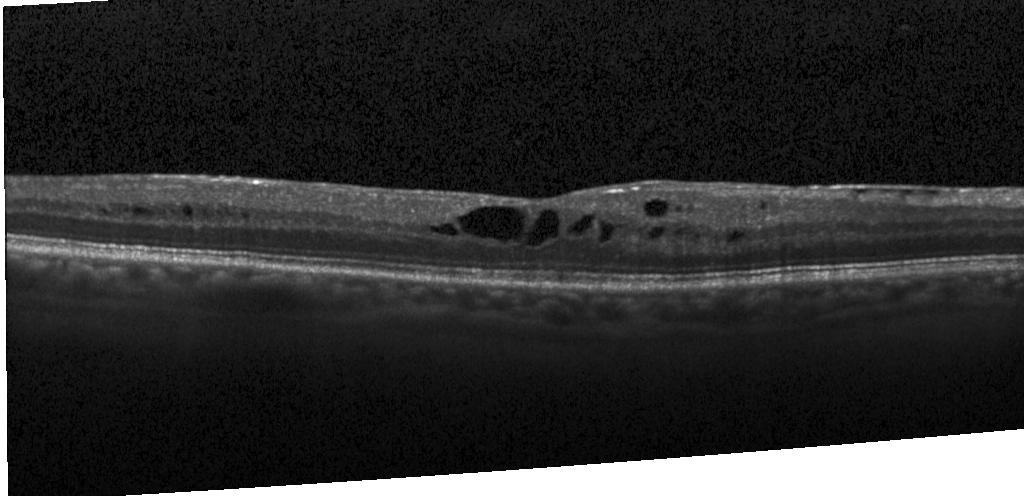

Retinal OCT B-scan; through the macula; Heidelberg Spectralis OCT system.
Finding: DME.